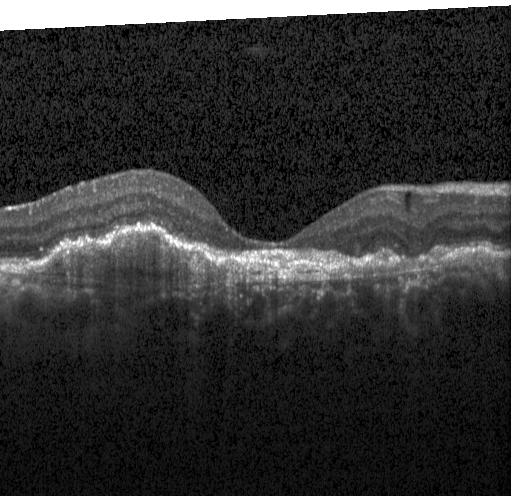
Retinal OCT cross-section. Impression: a choroidal neovascular membrane.